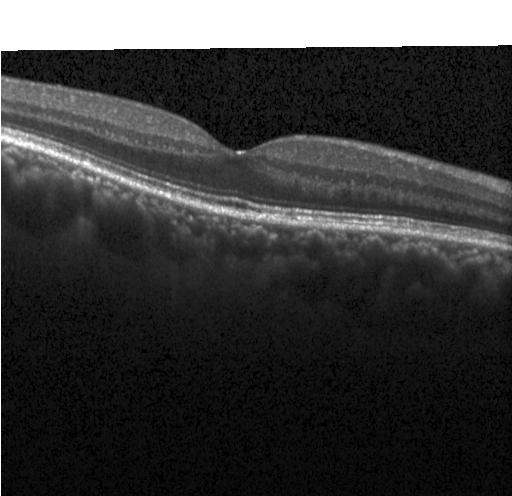

Heidelberg Spectralis · OCT line scan. This B-scan demonstrates no choroidal neovascularization, no diabetic macular edema, and no drusen.